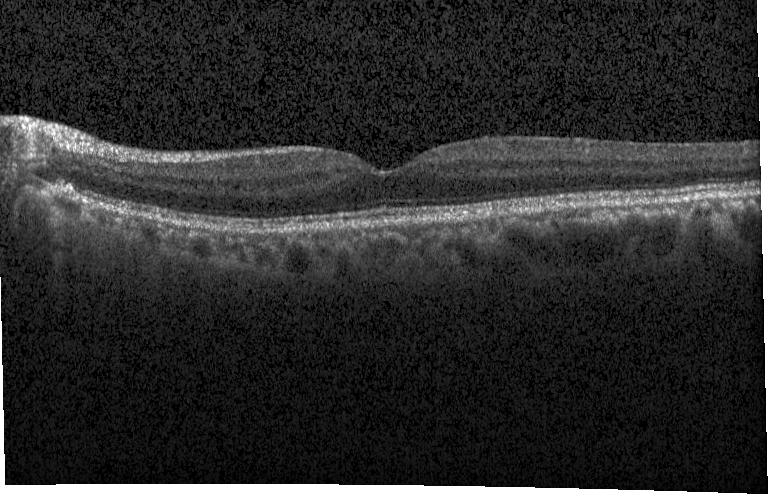

Heidelberg Spectralis. OCT B-scan. SD-OCT. Centered on the fovea.
Impression: no evidence of CNV, DME, or drusen.